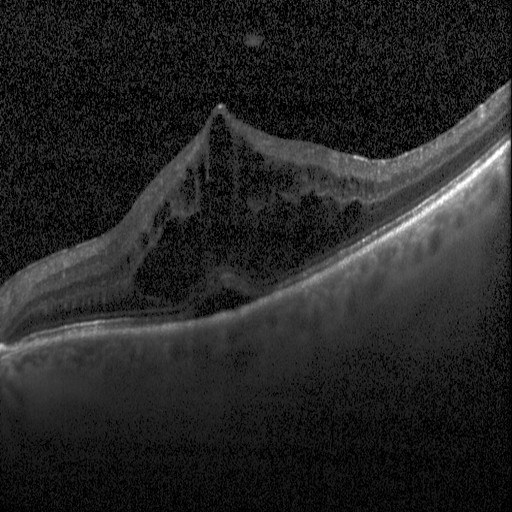
Macular OCT demonstrating DME.